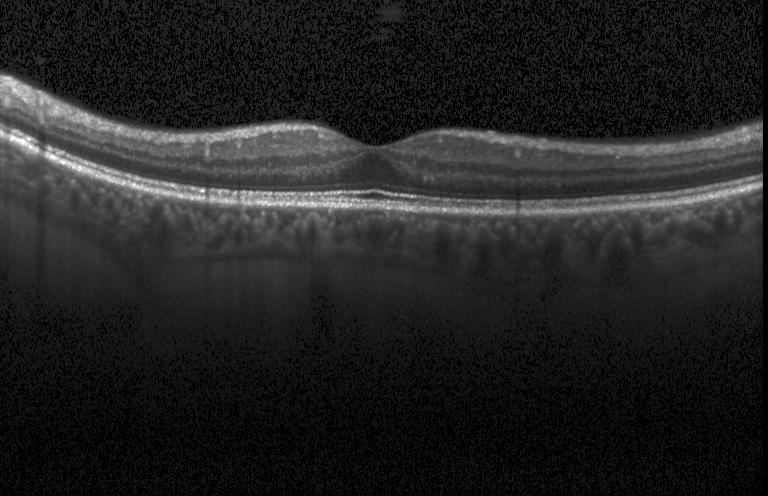 Optical coherence tomography scan
Neither choroidal neovascularization, diabetic macular edema, nor drusen.